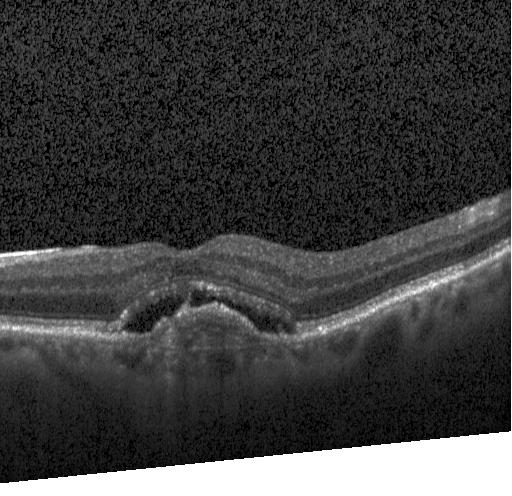

Through the macula. Retinal OCT cross-section — Finding: a choroidal neovascular membrane.